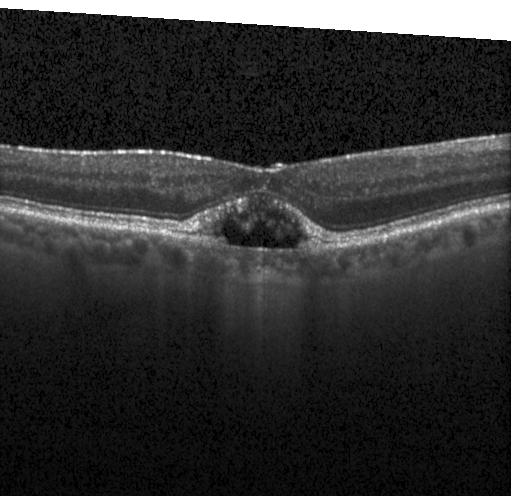 Spectral-domain OCT. Optical coherence tomography B-scan
OCT finding: choroidal neovascularization.